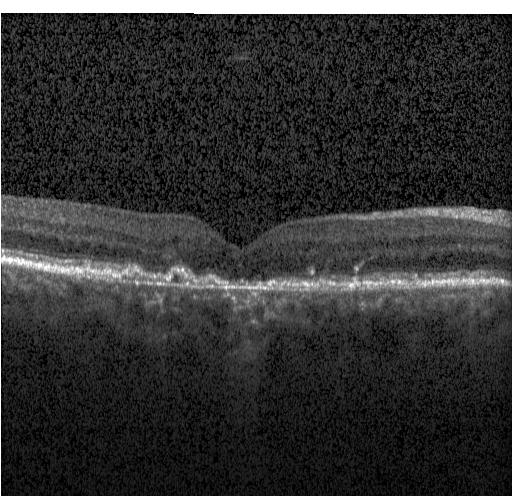 Retinal OCT B-scan; horizontal scan through the fovea; Heidelberg Spectralis. Macular OCT: CNV.